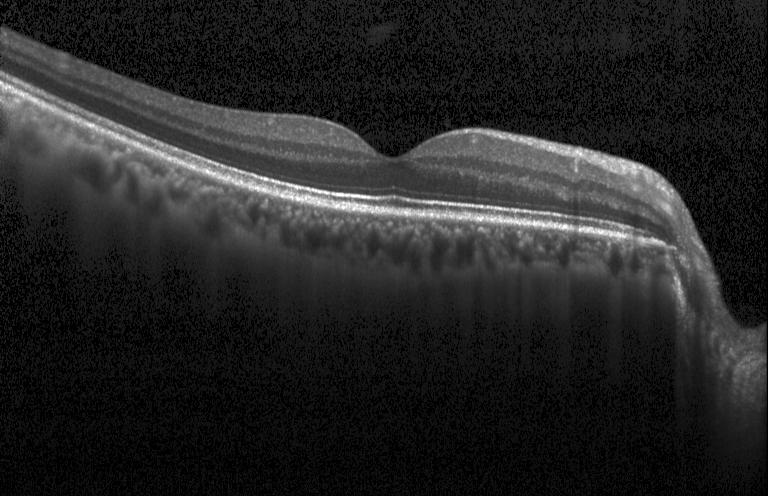
Acquired on a Heidelberg Spectralis; retinal OCT cross-section; SD-OCT. OCT finding: no CNV, no DME, and no drusen.